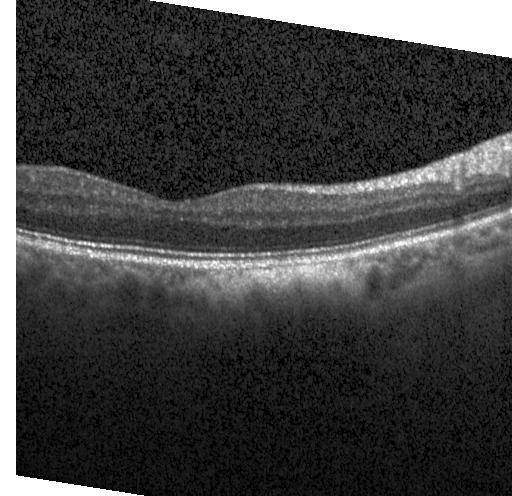 Heidelberg Spectralis OCT system. Horizontal scan through the fovea. SD-OCT. Retinal OCT cross-section — OCT finding: no evidence of choroidal neovascularization, diabetic macular edema, or drusen.